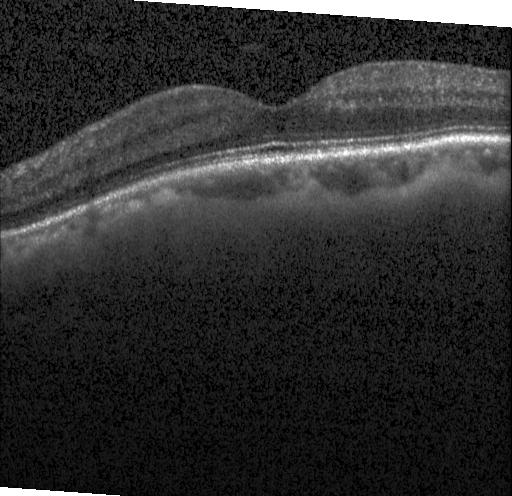 Optical coherence tomography B-scan. Spectral-domain OCT. Macular scan. Acquired on a Heidelberg Spectralis — The scan shows neither choroidal neovascularization, diabetic macular edema, nor drusen.